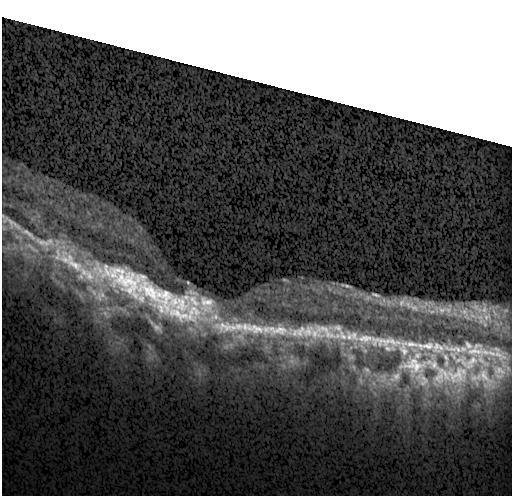 Spectral-domain optical coherence tomography, centered on the fovea, OCT line scan — The scan shows choroidal neovascularization.